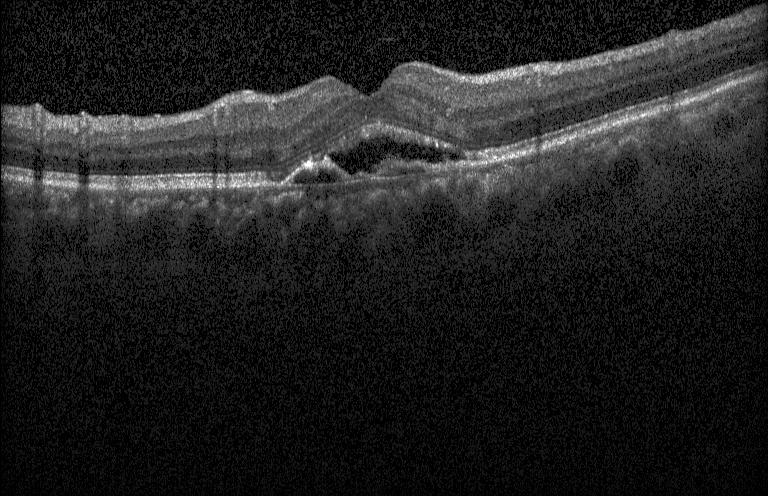

Acquired on a Heidelberg Spectralis, SD-OCT, optical coherence tomography scan. Diagnosis: a choroidal neovascular membrane.